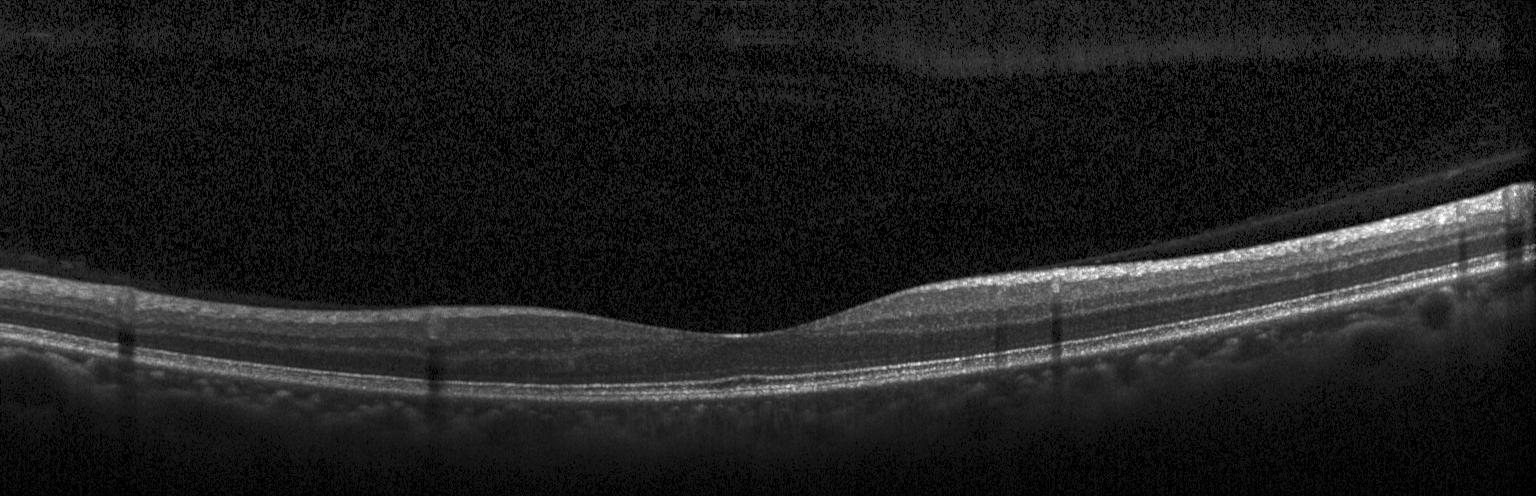
Instrument: Heidelberg Spectralis · OCT B-scan
Impression: no evidence of CNV, DME, or drusen.